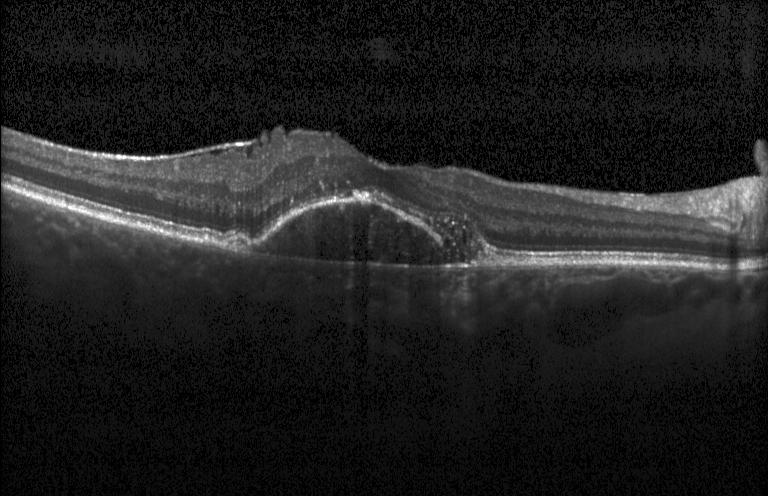
Optical coherence tomography scan · Heidelberg Spectralis OCT system.
This B-scan demonstrates a choroidal neovascular membrane.